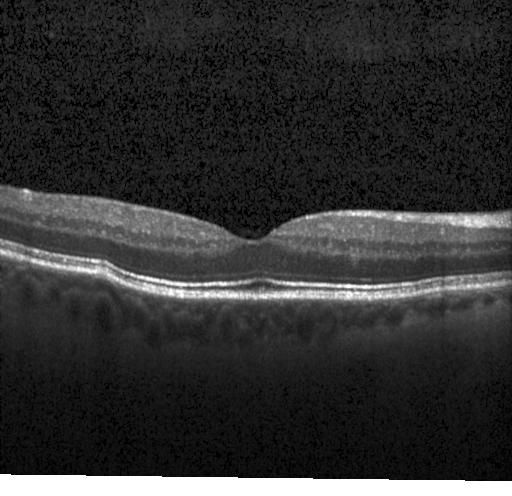

Horizontal scan through the fovea; Heidelberg Spectralis OCT system; OCT B-scan.
Diagnosis: no choroidal neovascularization, diabetic macular edema, or drusen.